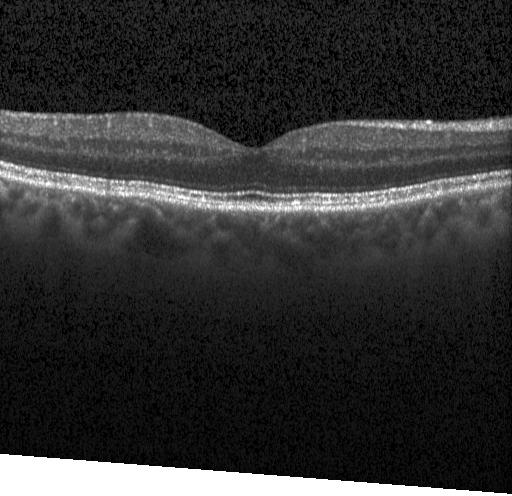
OCT line scan, fovea-centered, spectral-domain optical coherence tomography
Dx: no CNV, no DME, and no drusen.